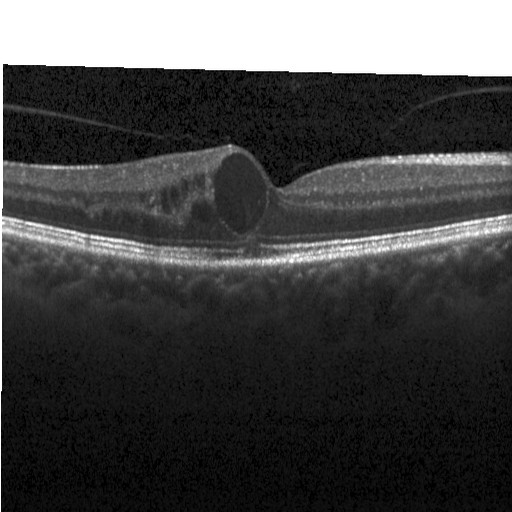
Through the macula, retinal OCT B-scan, acquired on a Heidelberg Spectralis.
Diagnosis: diabetic macular edema (DME).